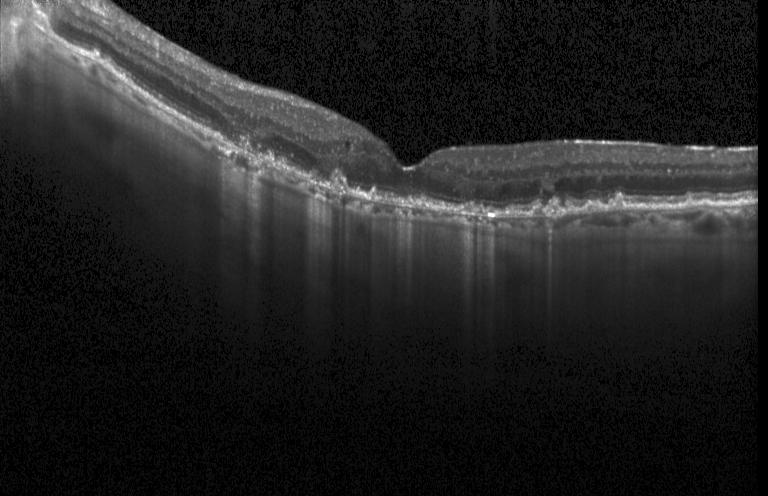 Optical coherence tomography B-scan, SD-OCT
Choroidal neovascularization.